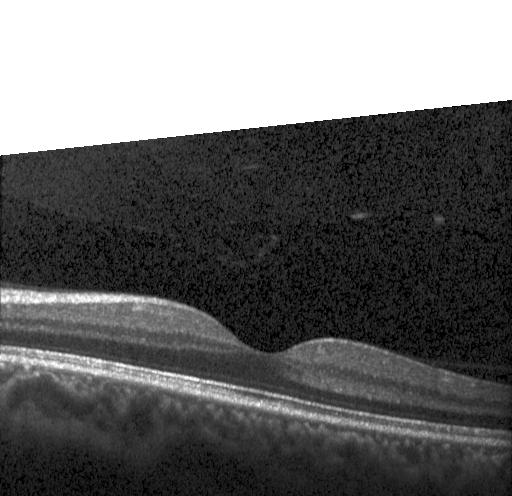 Diagnosis: no CNV, DME, or drusen.